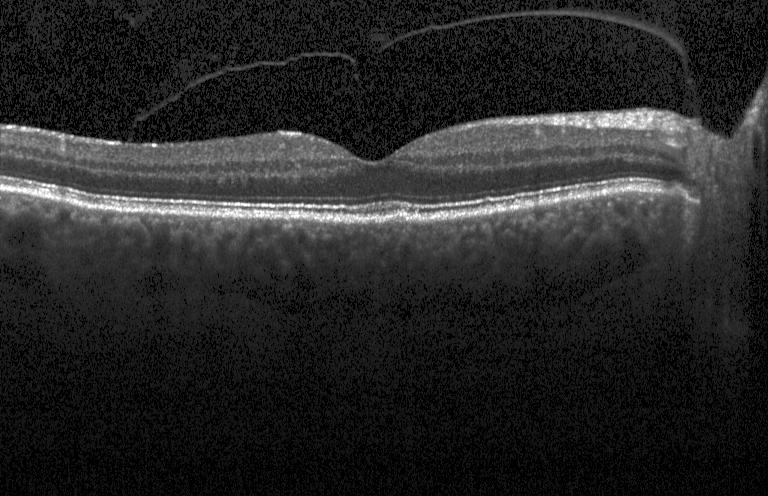

Through the macula, instrument: Heidelberg Spectralis, OCT B-scan.
The scan shows multiple drusen.